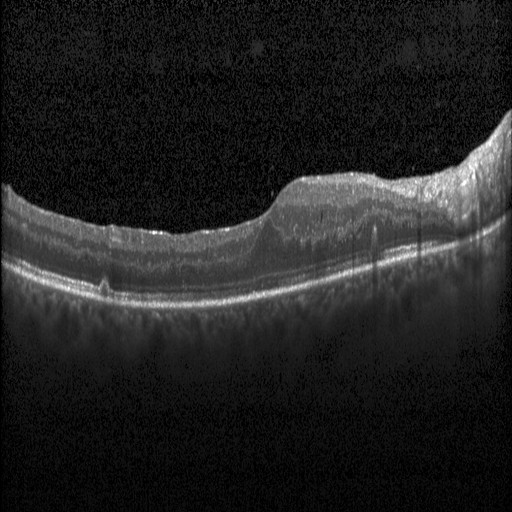 Retinal OCT B-scan; acquired on a Heidelberg Spectralis
OCT finding: diabetic macular edema.